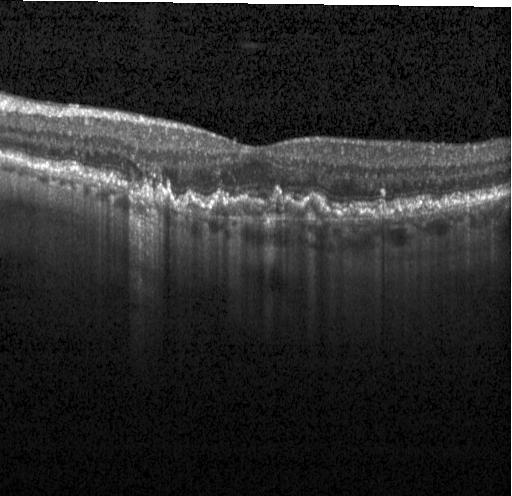
OCT B-scan, spectral-domain optical coherence tomography, acquired on a Heidelberg Spectralis, fovea-centered.
Dx: CNV.